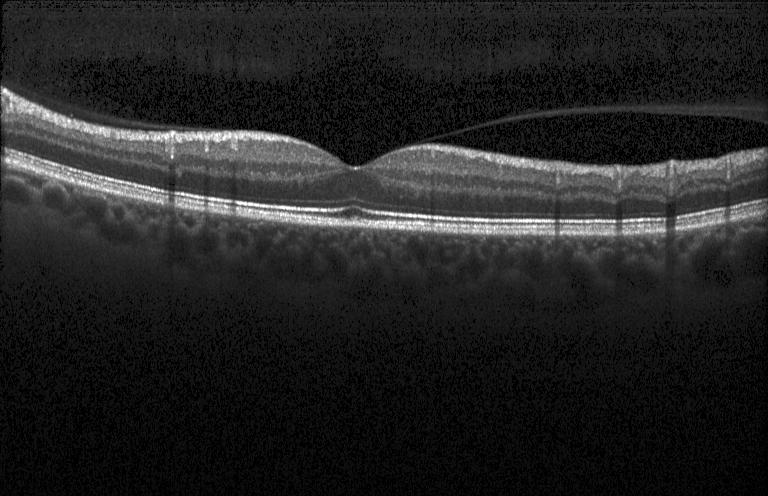

Dx: no evidence of CNV, DME, or drusen.